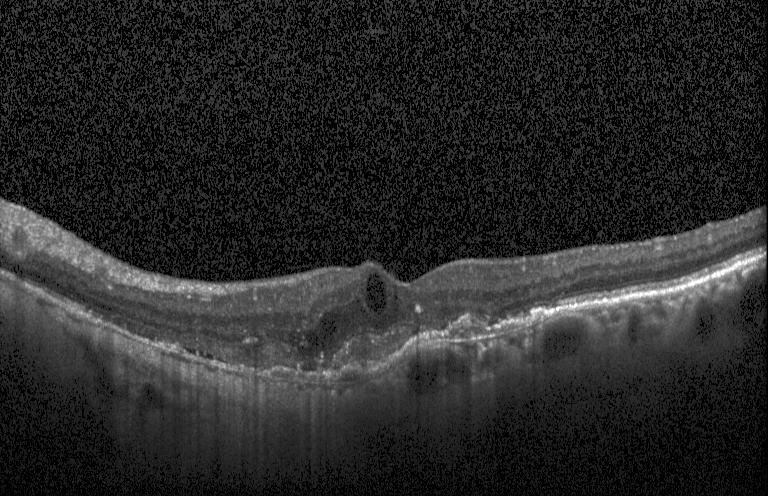 Spectral-domain optical coherence tomography; Heidelberg Spectralis OCT system; macular scan; retinal OCT cross-section. Assessment: CNV.